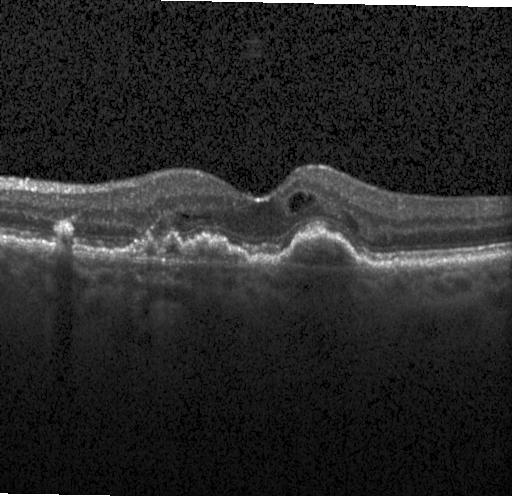

OCT finding: choroidal neovascularization (CNV).